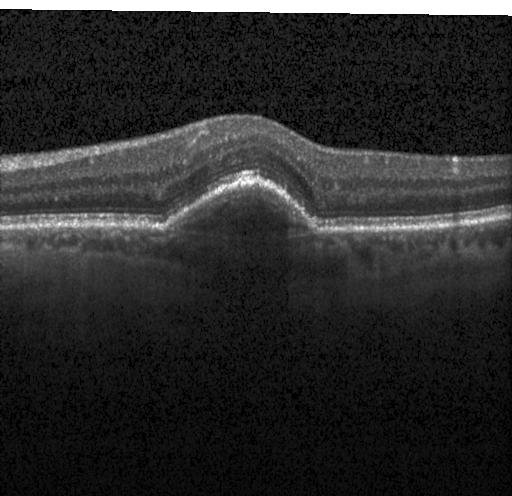 Retinal OCT cross-section · acquired on a Heidelberg Spectralis · spectral-domain OCT — OCT finding: a choroidal neovascular membrane.